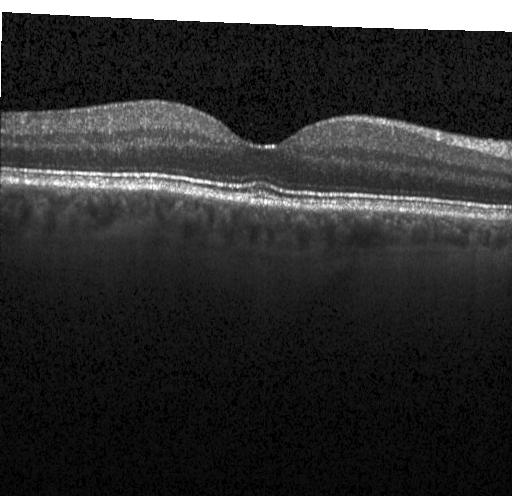
Heidelberg Spectralis; SD-OCT; retinal OCT cross-section — Assessment: neither choroidal neovascularization, diabetic macular edema, nor drusen.